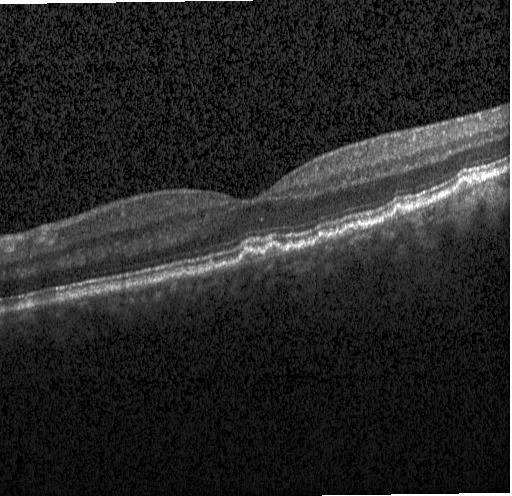
Optical coherence tomography scan; spectral-domain OCT; fovea-centered
Impression: drusen.